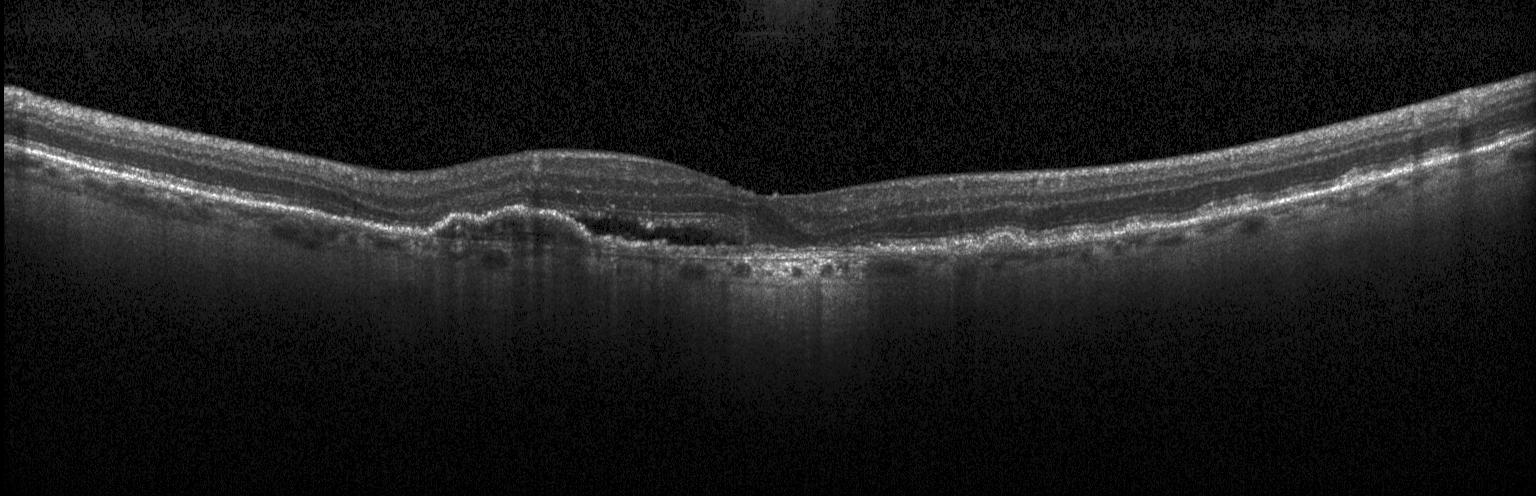

OCT B-scan — Dx: a choroidal neovascular membrane.